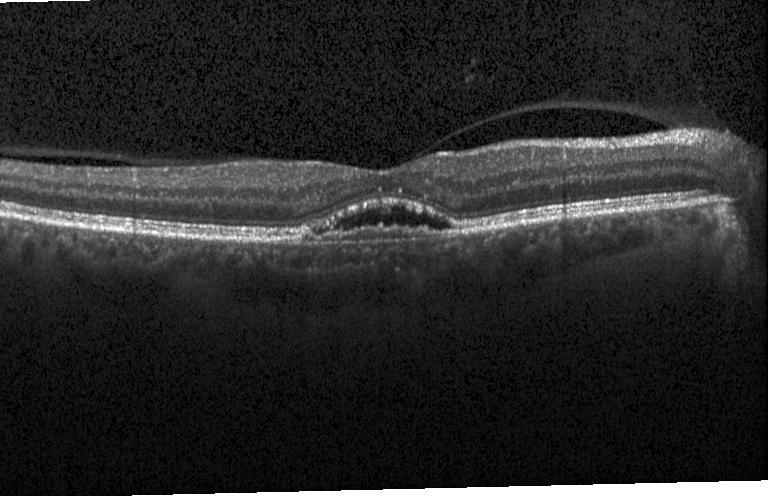 Heidelberg Spectralis OCT system; retinal OCT B-scan; spectral-domain OCT — Diagnosis: choroidal neovascularization.